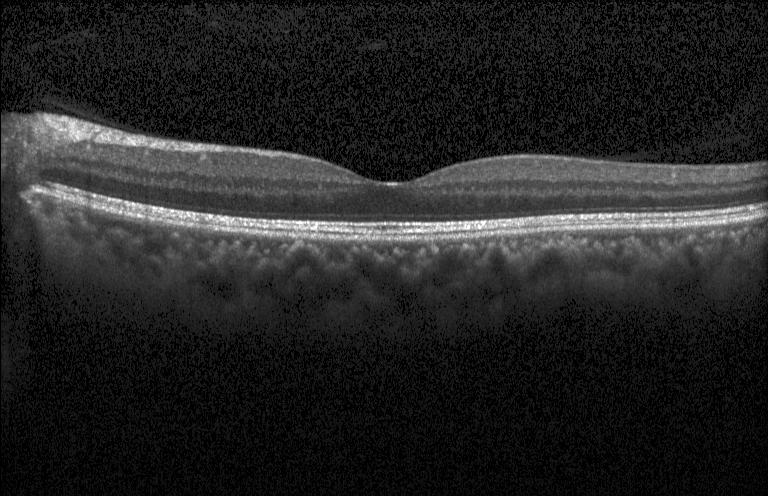
Retinal OCT B-scan. OCT finding: no evidence of choroidal neovascularization, diabetic macular edema, or drusen.